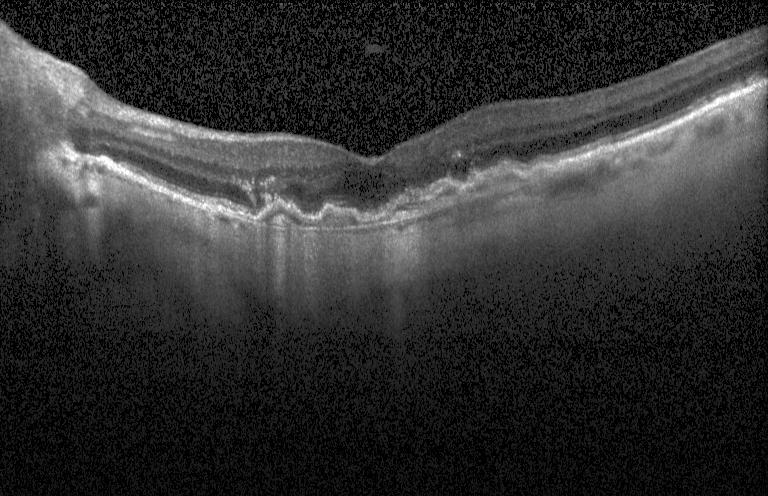 Spectral-domain OCT; instrument: Heidelberg Spectralis; macular scan; OCT B-scan — This B-scan demonstrates choroidal neovascularization (CNV).